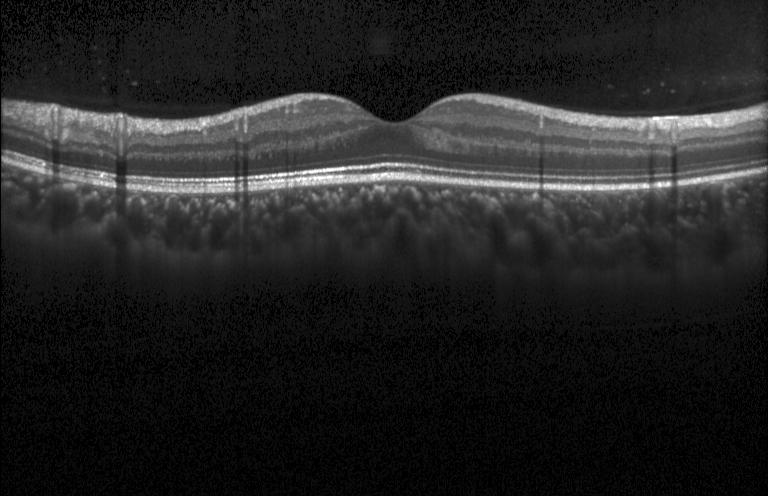

Optical coherence tomography B-scan — Diagnosis: neither choroidal neovascularization, diabetic macular edema, nor drusen.